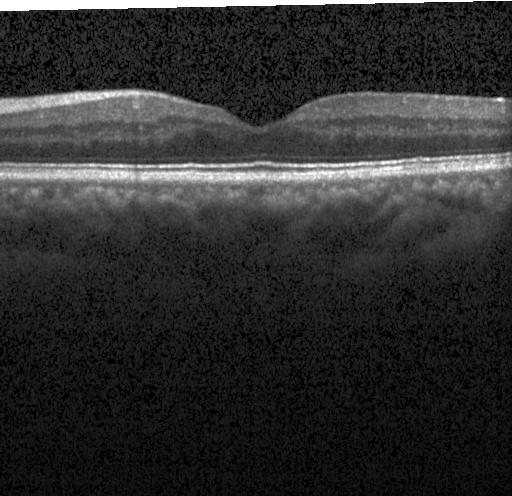

Horizontal scan through the fovea · retinal OCT B-scan · spectral-domain optical coherence tomography — Finding: no CNV, no DME, and no drusen.